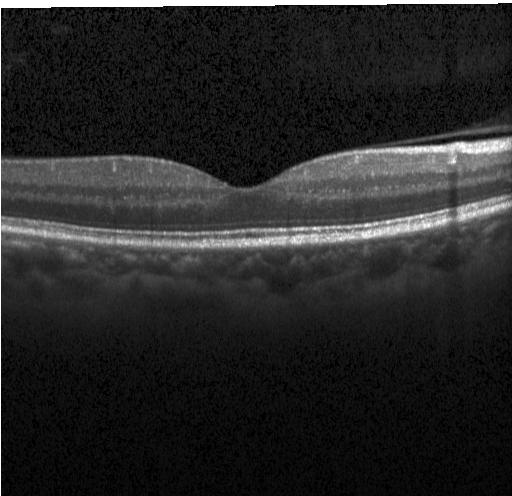
Centered on the fovea · OCT line scan · instrument: Heidelberg Spectralis. This B-scan demonstrates no choroidal neovascularization, diabetic macular edema, or drusen.